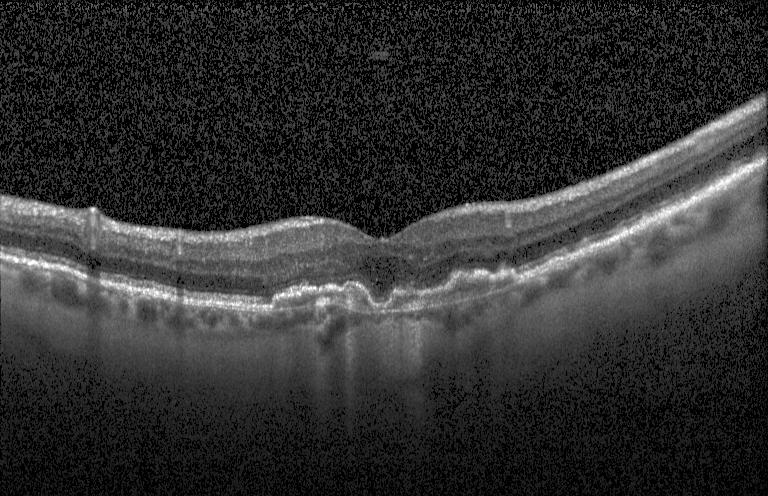 Retinal OCT cross-section, macular scan.
Assessment: choroidal neovascularization (CNV).